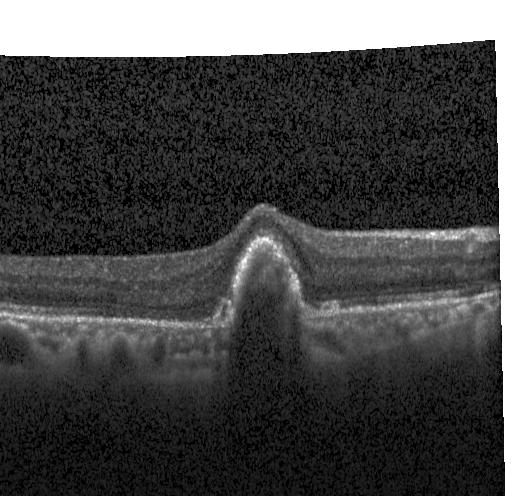 Centered on the fovea. Retinal OCT cross-section — Finding: a choroidal neovascular membrane.